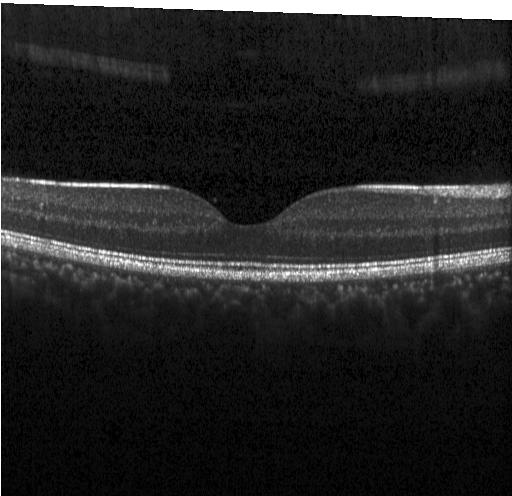
Finding: no choroidal neovascularization, no diabetic macular edema, and no drusen.